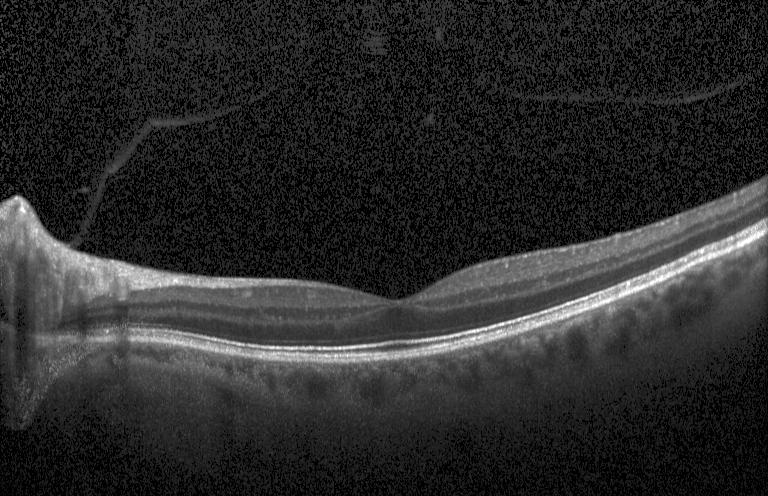 Fovea-centered. Optical coherence tomography scan. This B-scan demonstrates neither choroidal neovascularization, diabetic macular edema, nor drusen.